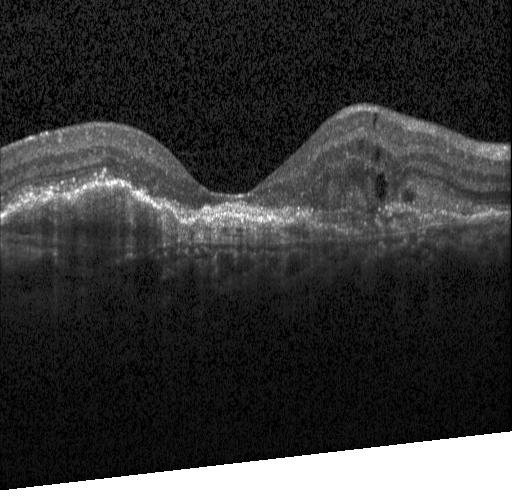

Retinal OCT cross-section — Dx: a choroidal neovascular membrane.